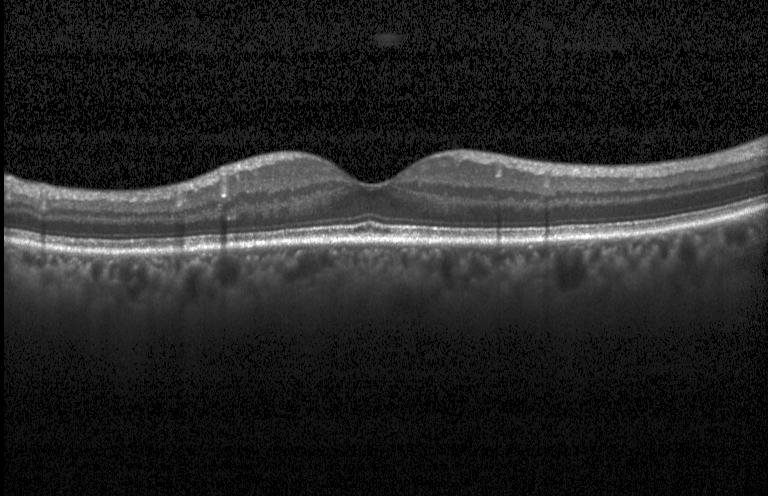
Spectral-domain OCT; optical coherence tomography scan; macular scan; acquired on a Heidelberg Spectralis. Assessment: no choroidal neovascularization, no diabetic macular edema, and no drusen.